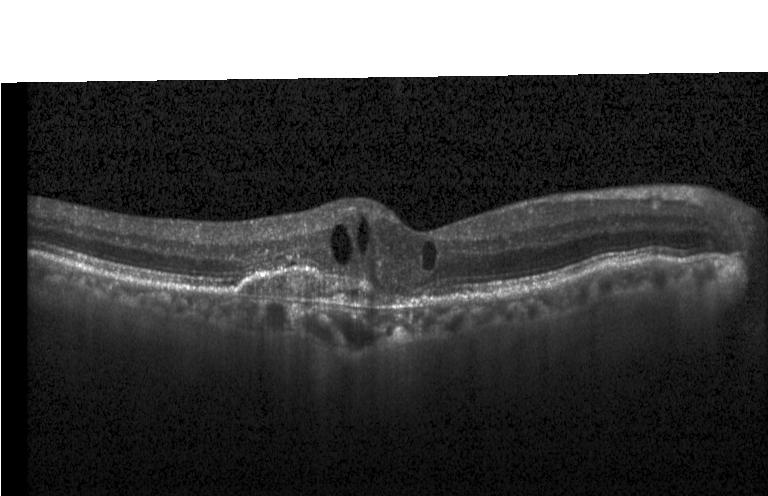

OCT line scan. Macular OCT: choroidal neovascularization (CNV).